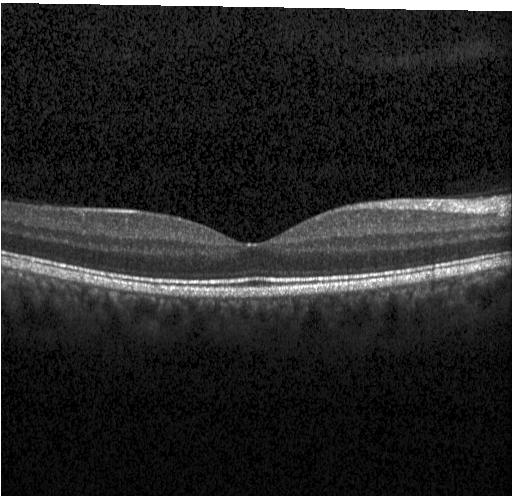

Finding: no choroidal neovascularization, diabetic macular edema, or drusen.